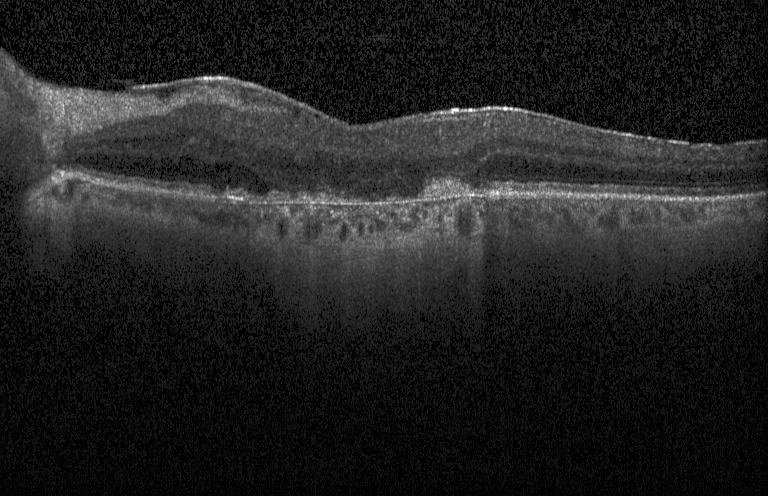

Heidelberg Spectralis, OCT line scan.
Finding: CNV.